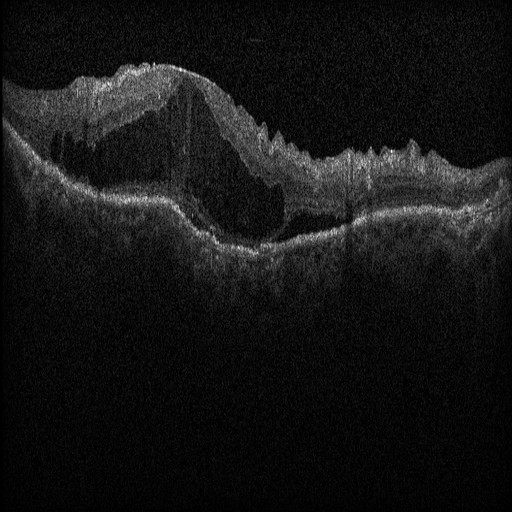
Spectral-domain OCT. Retinal OCT cross-section. Instrument: Heidelberg Spectralis. Impression: diabetic macular edema.